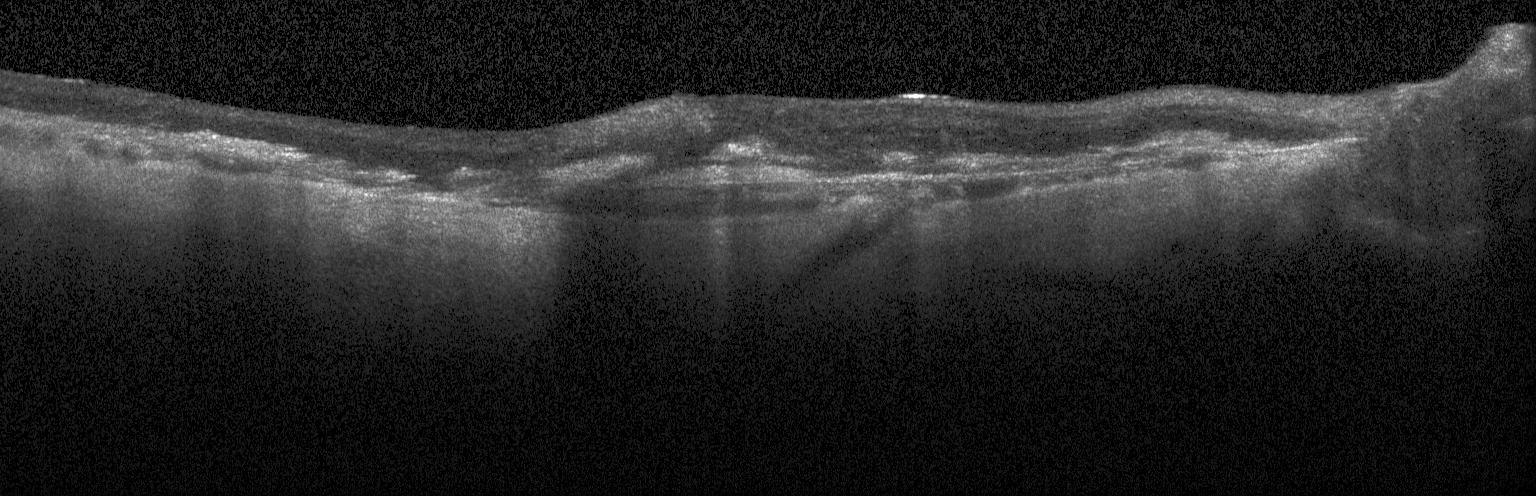
Retinal OCT cross-section.
Assessment: a choroidal neovascular membrane.